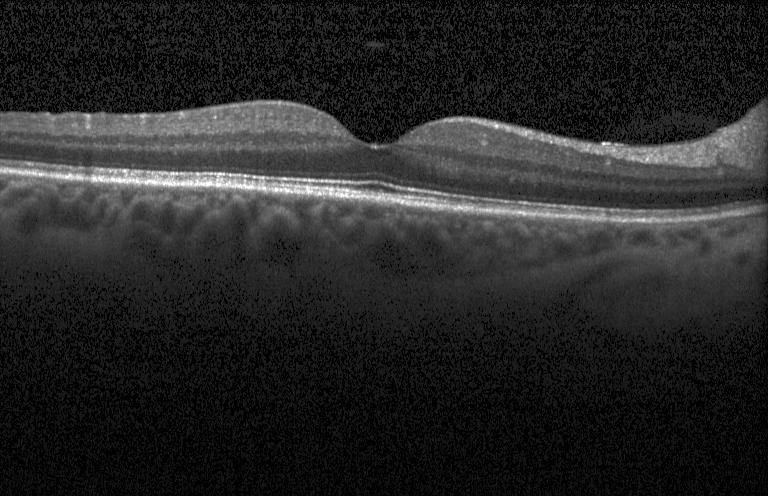

Retinal OCT B-scan
Impression: neither choroidal neovascularization, diabetic macular edema, nor drusen.